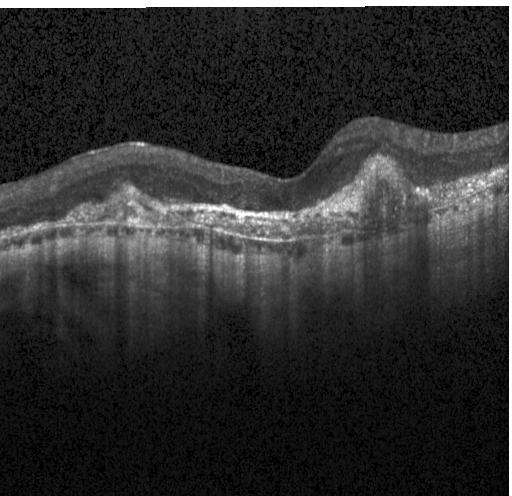
Spectral-domain OCT, centered on the fovea, retinal OCT cross-section, Heidelberg Spectralis OCT system.
Assessment: choroidal neovascularization (CNV).